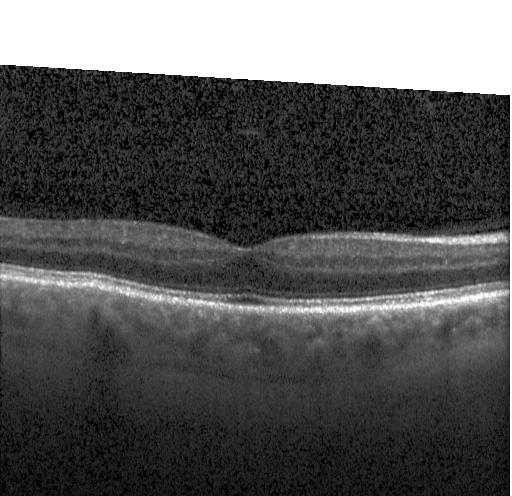

The scan shows no choroidal neovascularization, no diabetic macular edema, and no drusen.